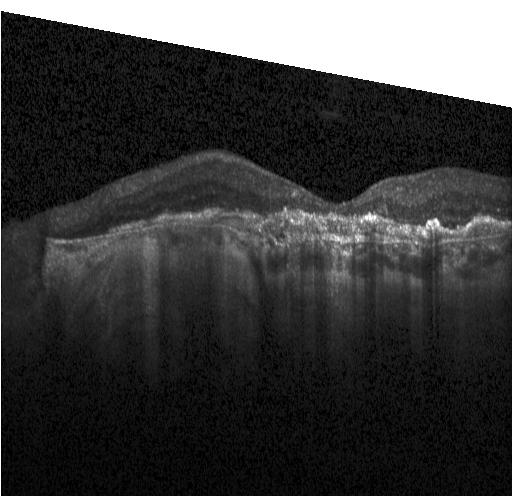 Diagnosis: a choroidal neovascular membrane.